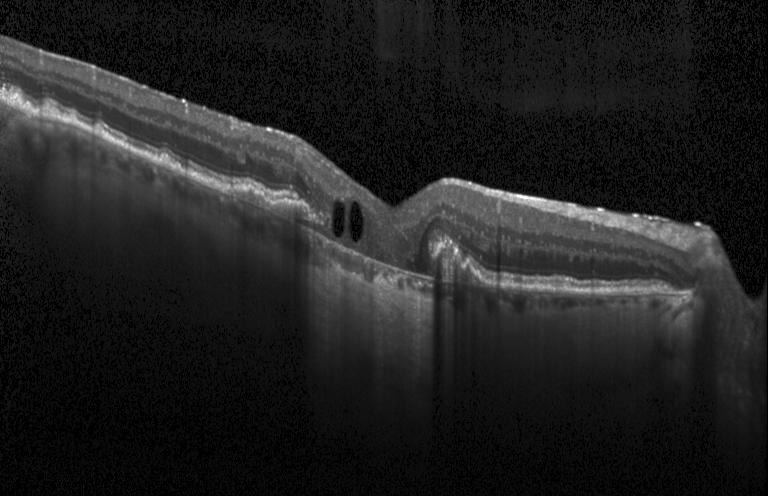

OCT B-scan. Spectral-domain OCT.
A choroidal neovascular membrane.